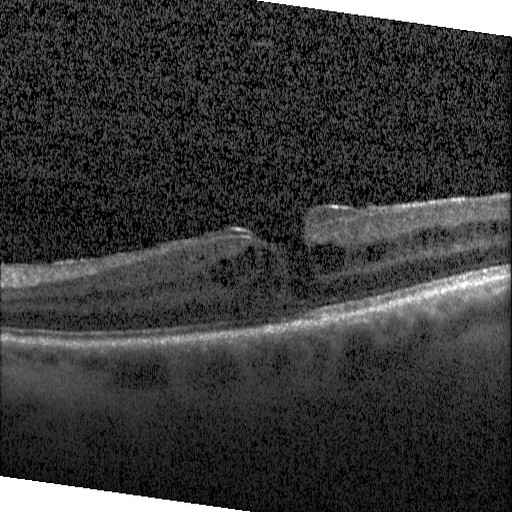

Assessment: diabetic macular edema (DME).